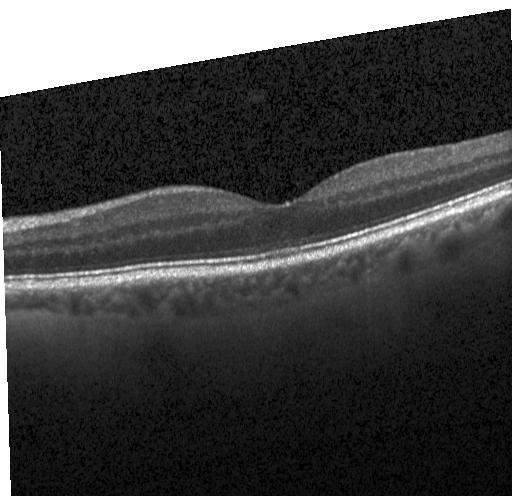 Optical coherence tomography scan. Instrument: Heidelberg Spectralis. Spectral-domain OCT — Finding: neither CNV, DME, nor drusen.